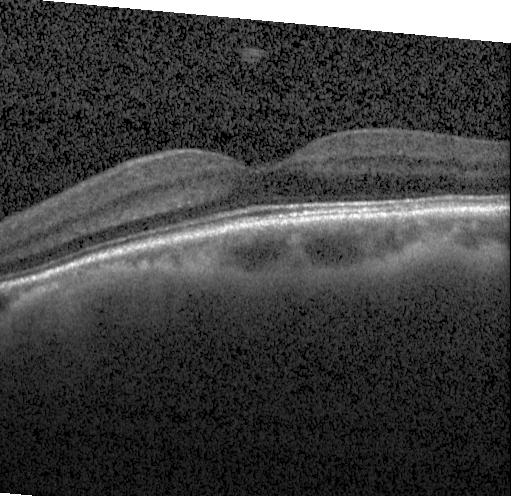
Heidelberg Spectralis; macular scan; optical coherence tomography scan. Impression: neither choroidal neovascularization, diabetic macular edema, nor drusen.